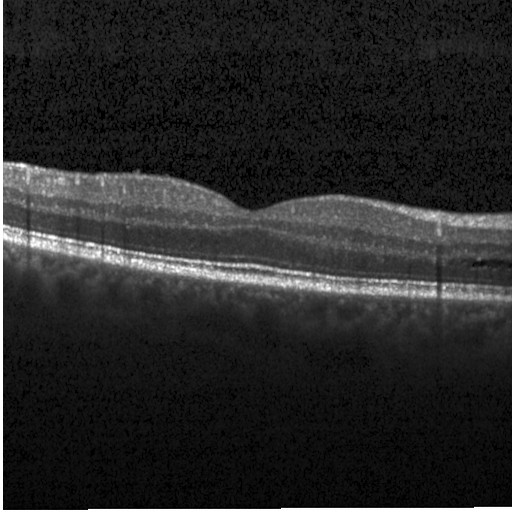
Fovea-centered; spectral-domain optical coherence tomography; Heidelberg Spectralis; optical coherence tomography B-scan.
Impression: diabetic macular edema.